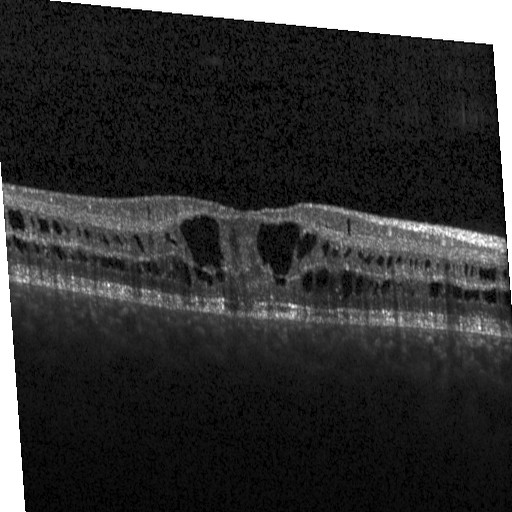

OCT B-scan
Finding: diabetic macular edema.